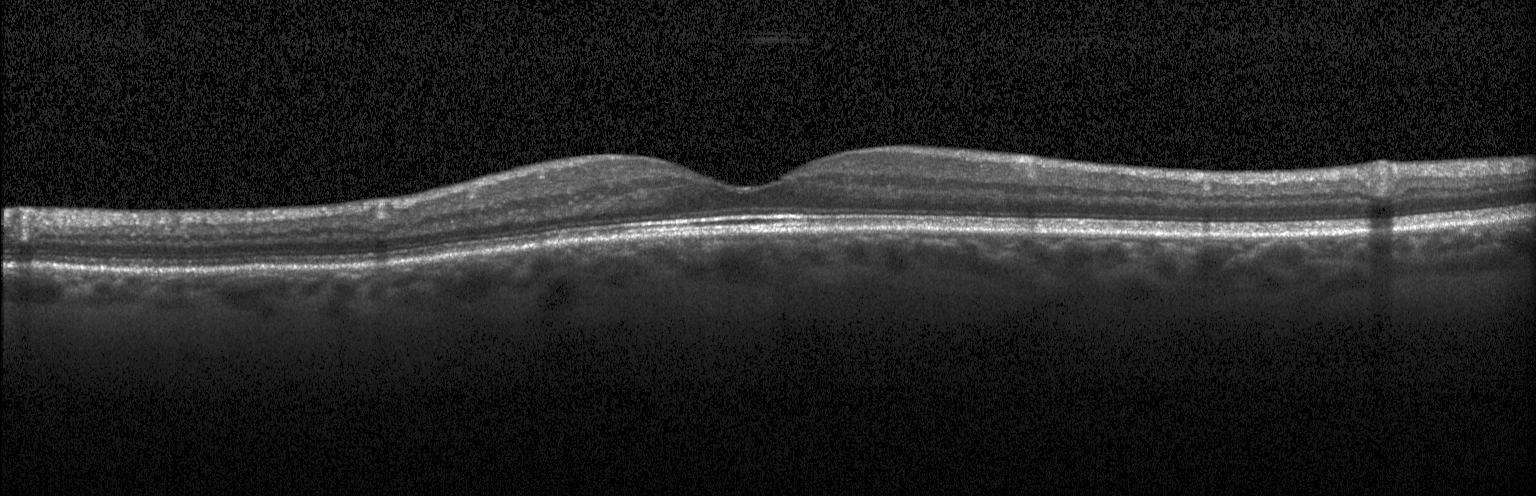 Finding: no evidence of choroidal neovascularization, diabetic macular edema, or drusen.